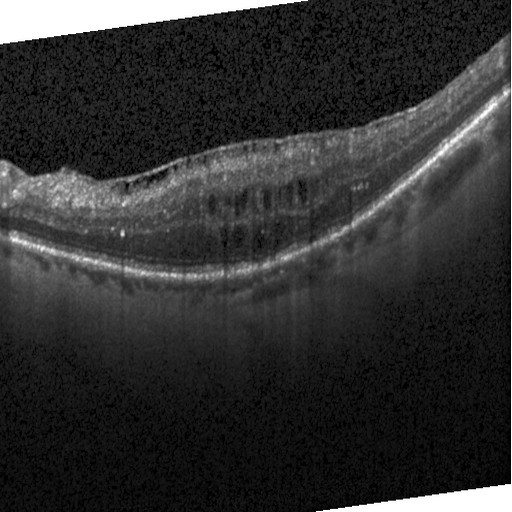 Horizontal scan through the fovea, instrument: Heidelberg Spectralis, spectral-domain OCT, optical coherence tomography scan — Finding: diabetic macular edema.